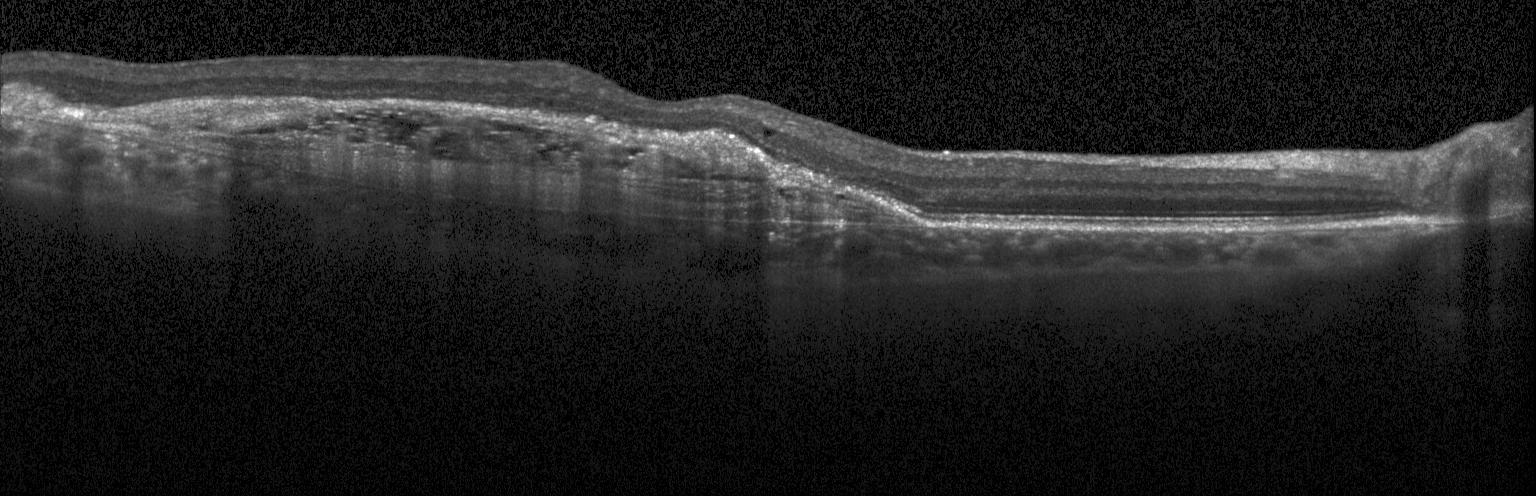
OCT finding: a choroidal neovascular membrane.